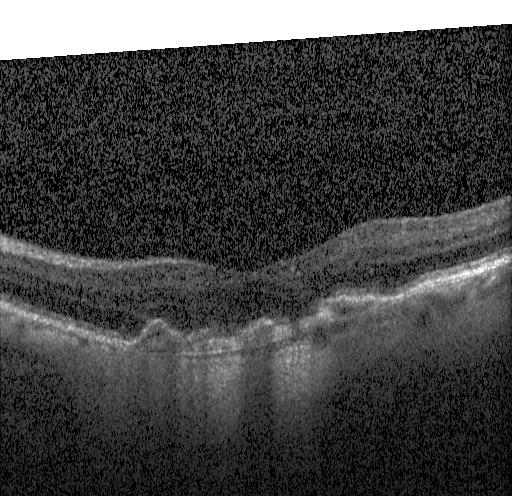 Retinal OCT cross-section showing a choroidal neovascular membrane.